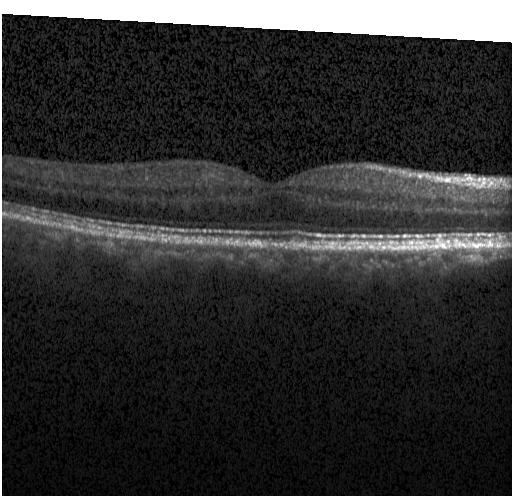
Dx: no choroidal neovascularization, no diabetic macular edema, and no drusen.